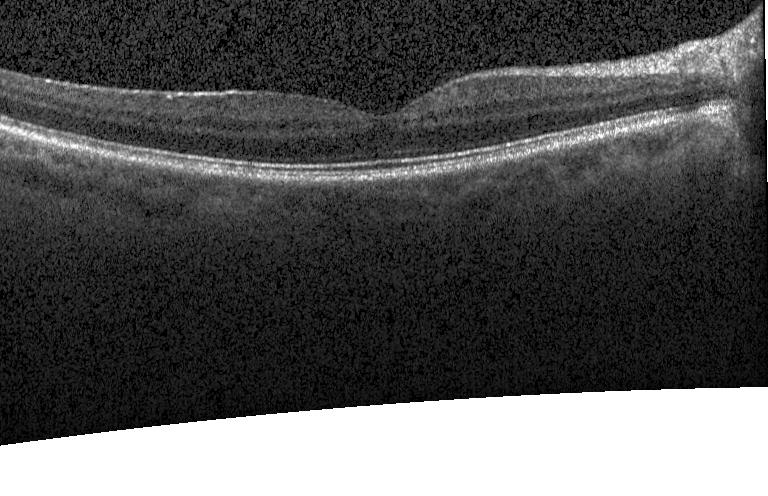

OCT B-scan showing no choroidal neovascularization, no diabetic macular edema, and no drusen.